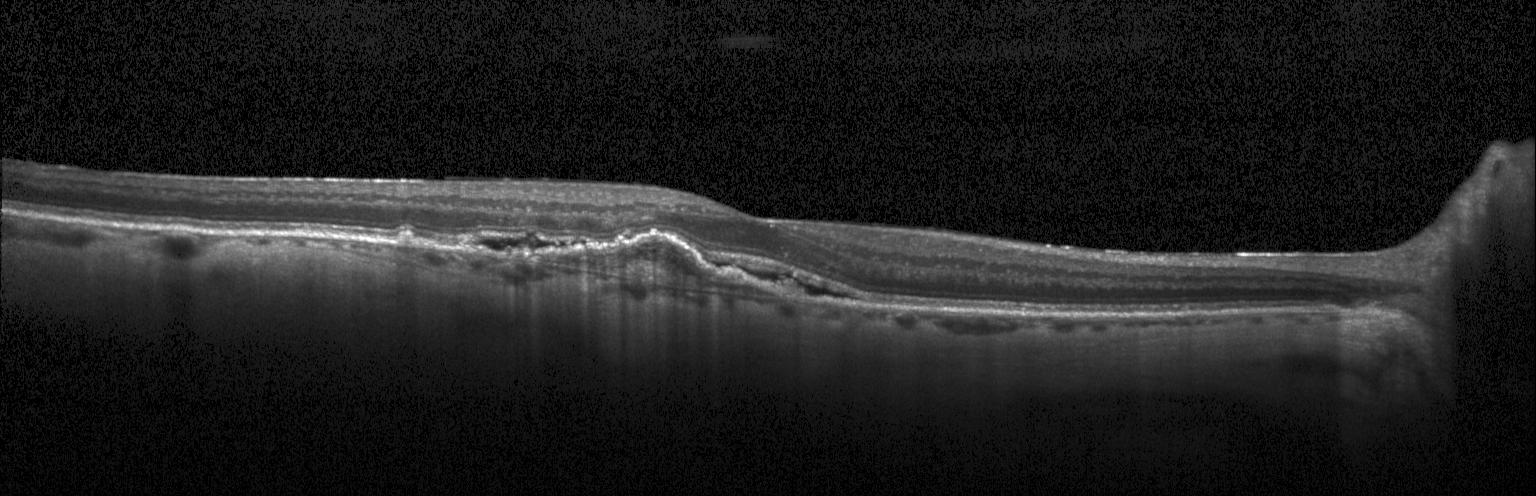 OCT line scan, spectral-domain optical coherence tomography — The scan shows a choroidal neovascular membrane.